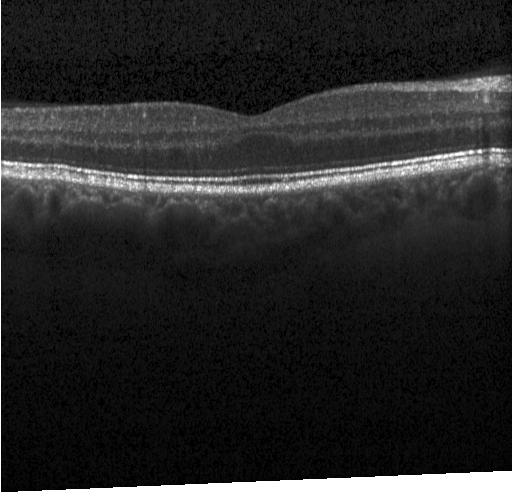
Retinal OCT B-scan; centered on the fovea
Macular OCT: no CNV, DME, or drusen.